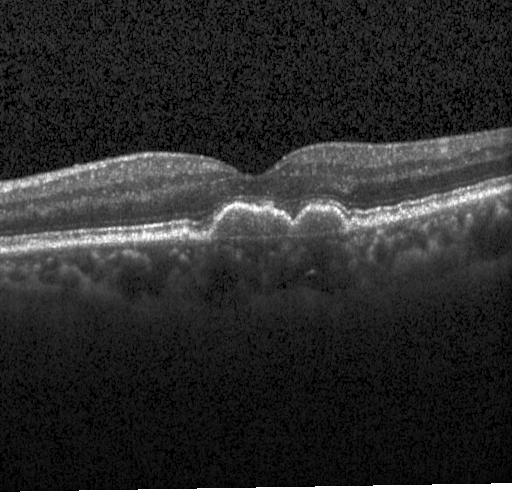 Heidelberg Spectralis OCT system · spectral-domain OCT · macular scan · retinal OCT cross-section.
Diagnosis: sub-RPE drusenoid deposits.